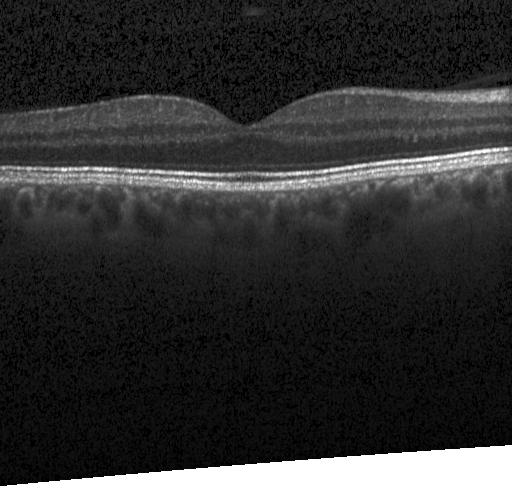

Spectral-domain optical coherence tomography; macular scan; optical coherence tomography B-scan.
Impression: no CNV, no DME, and no drusen.